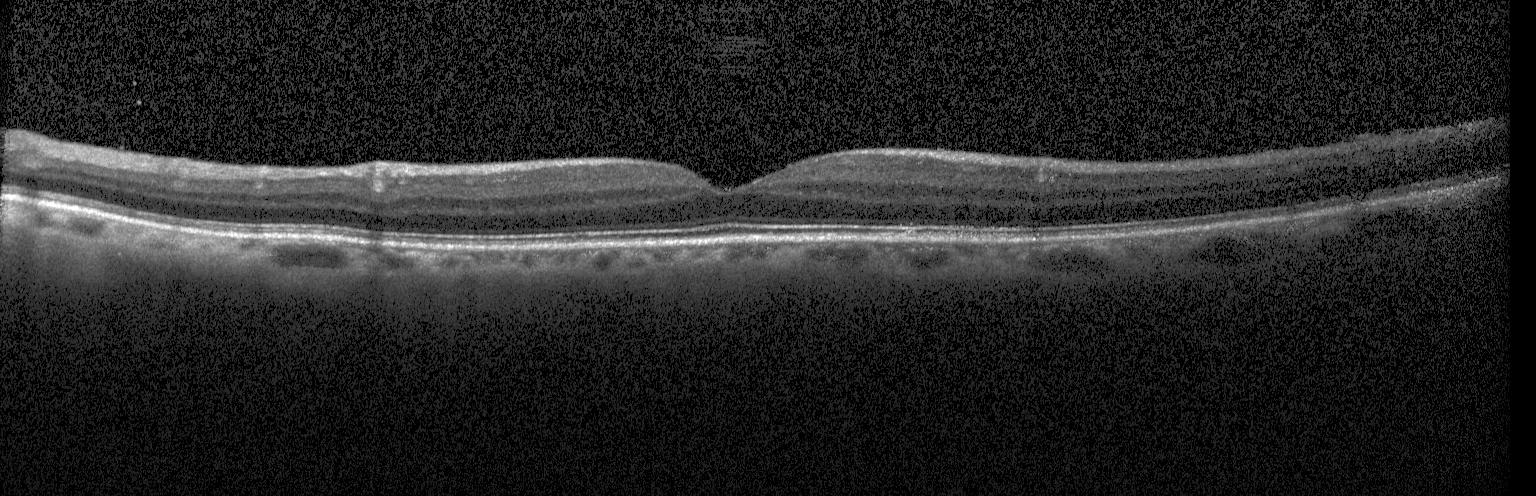 Finding: no CNV, no DME, and no drusen.